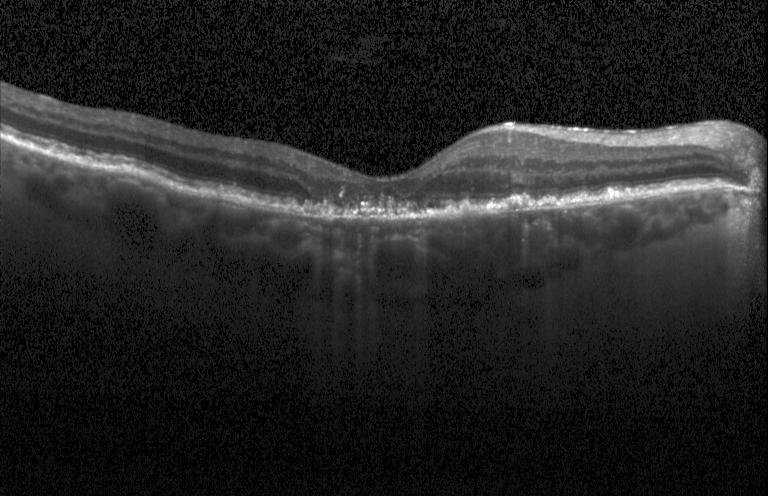 Retinal OCT cross-section. Horizontal scan through the fovea. Heidelberg Spectralis OCT system. Spectral-domain optical coherence tomography. Choroidal neovascularization.